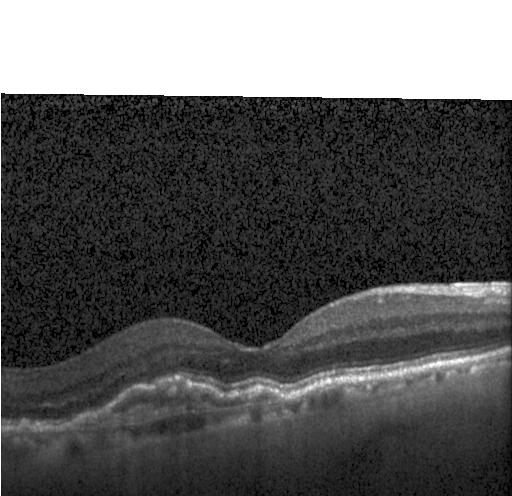 Heidelberg Spectralis; optical coherence tomography B-scan — Diagnosis: choroidal neovascularization.